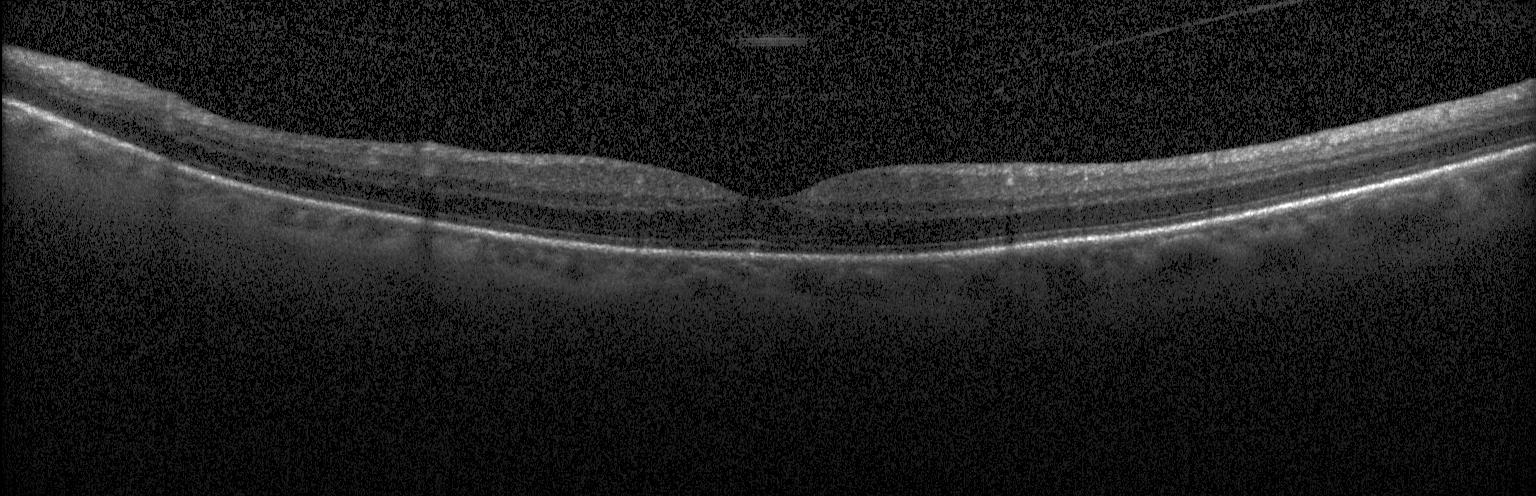
Retinal OCT cross-section. Heidelberg Spectralis OCT system.
Impression: no evidence of CNV, DME, or drusen.